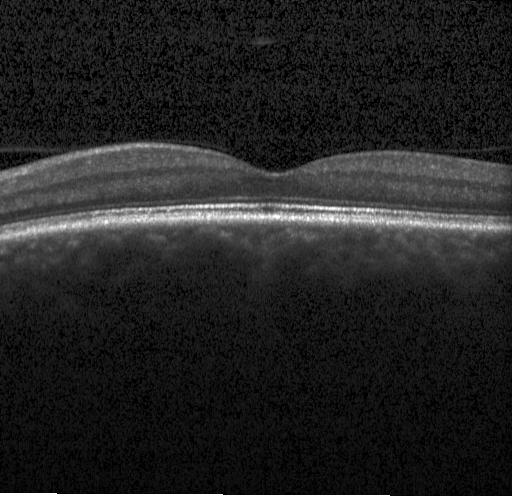 Fovea-centered · spectral-domain optical coherence tomography · Heidelberg Spectralis OCT system · retinal OCT cross-section
Macular OCT: neither choroidal neovascularization, diabetic macular edema, nor drusen.